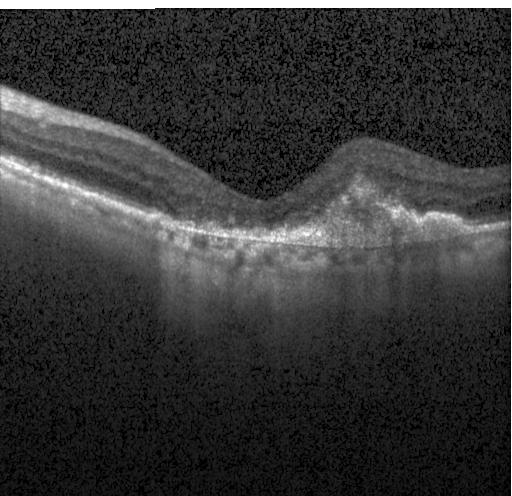
Macular scan; optical coherence tomography scan; spectral-domain optical coherence tomography
Assessment: choroidal neovascularization.